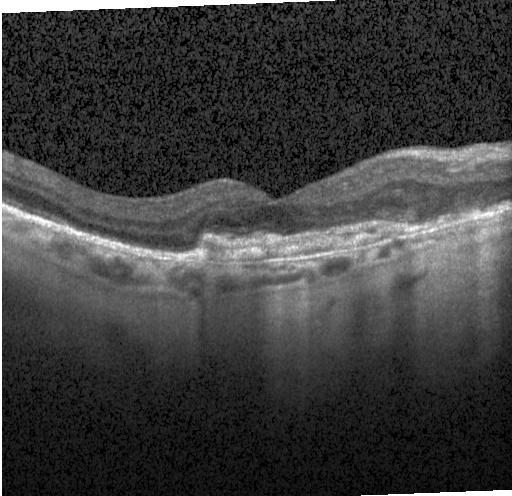

Finding: a choroidal neovascular membrane.